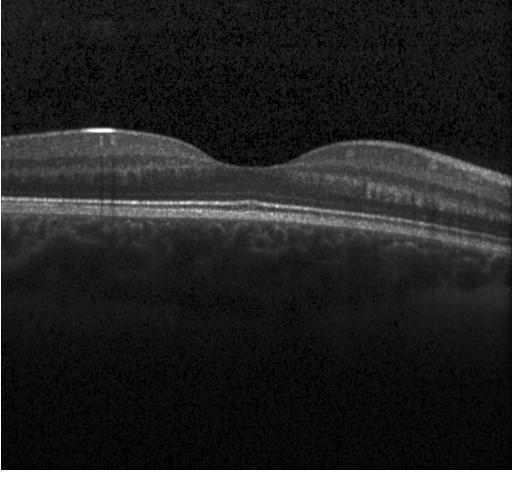

Retinal OCT B-scan; through the macula — Finding: no CNV, no DME, and no drusen.